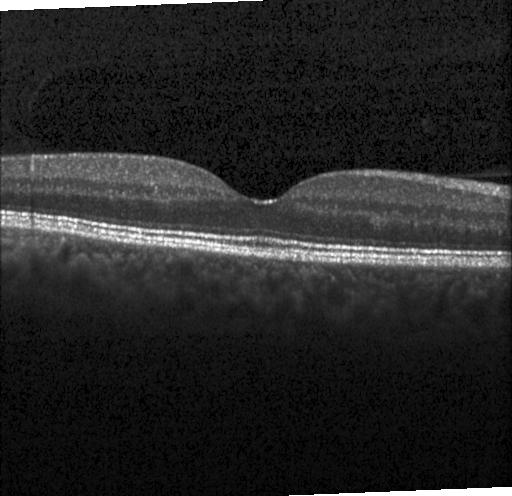 Acquired on a Heidelberg Spectralis. SD-OCT. Optical coherence tomography scan. Horizontal scan through the fovea — Impression: neither CNV, DME, nor drusen.